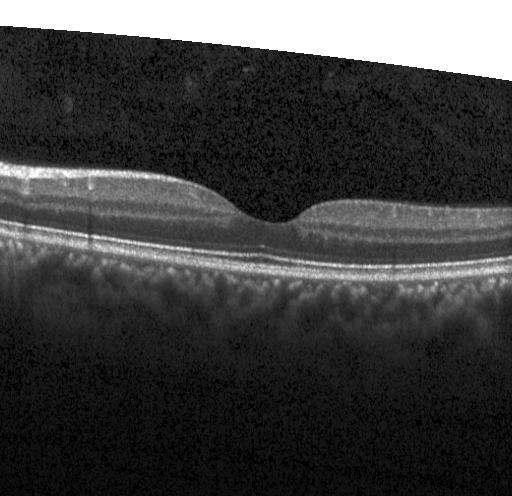

Retinal OCT B-scan; Heidelberg Spectralis
Assessment: neither choroidal neovascularization, diabetic macular edema, nor drusen.